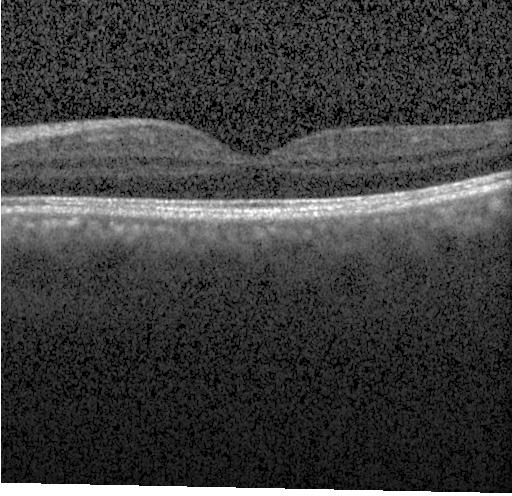
Instrument: Heidelberg Spectralis. Retinal OCT B-scan — Macular OCT: no choroidal neovascularization, diabetic macular edema, or drusen.